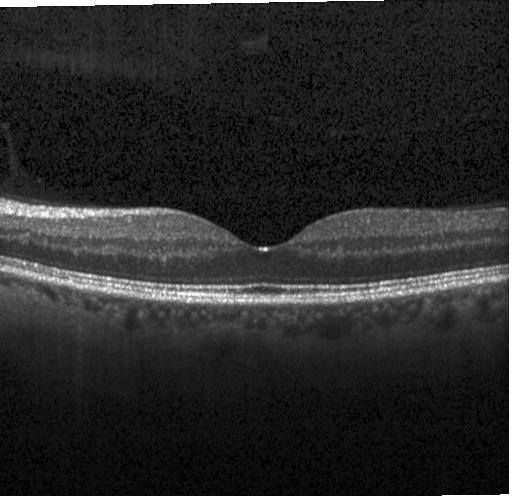 Dx: neither choroidal neovascularization, diabetic macular edema, nor drusen.